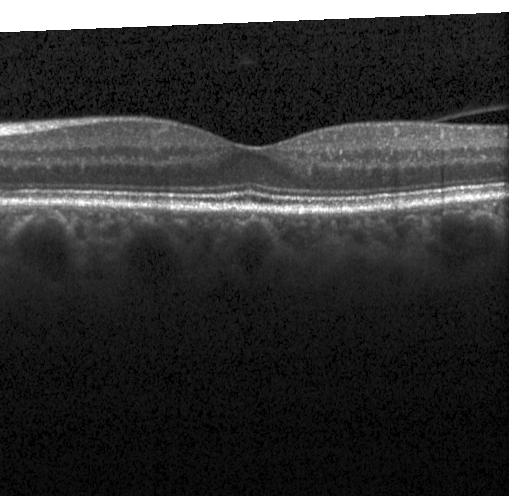

Optical coherence tomography scan · horizontal scan through the fovea · spectral-domain optical coherence tomography
Impression: no CNV, DME, or drusen.